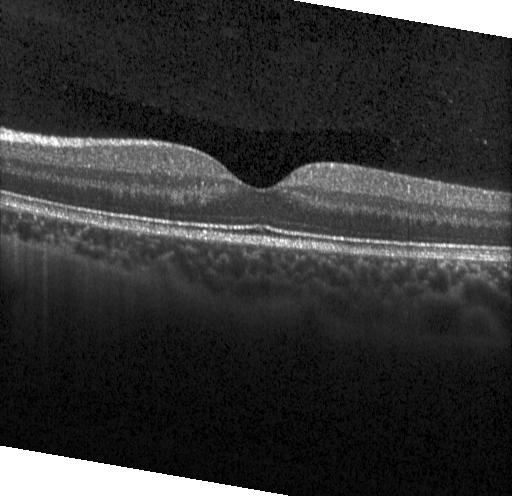

OCT line scan, acquired on a Heidelberg Spectralis
Assessment: no choroidal neovascularization, diabetic macular edema, or drusen.